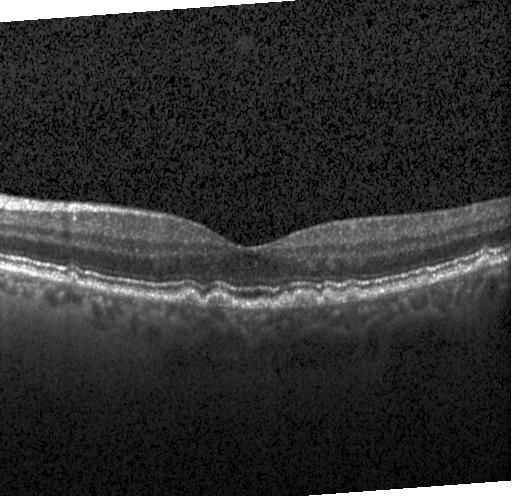 Instrument: Heidelberg Spectralis, spectral-domain OCT, optical coherence tomography scan
Diagnosis: sub-RPE drusenoid deposits.